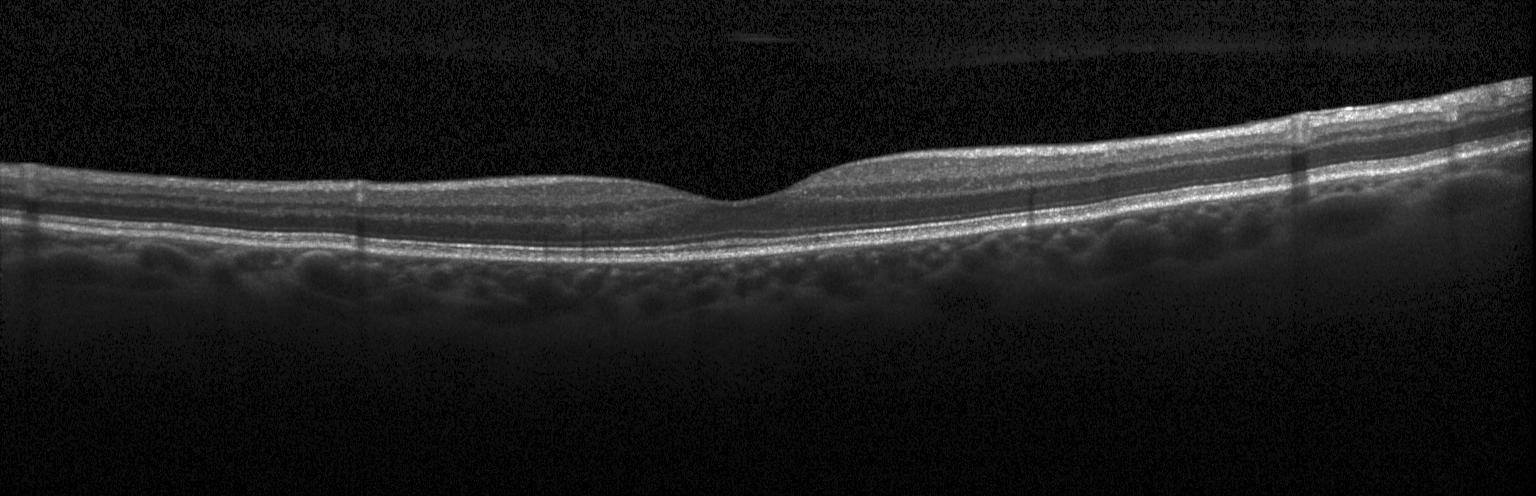

Optical coherence tomography B-scan.
Impression: no evidence of choroidal neovascularization, diabetic macular edema, or drusen.